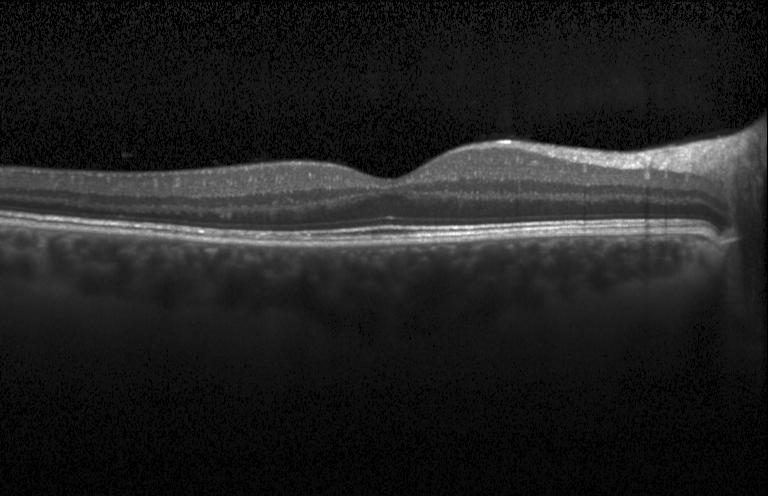 Finding: no choroidal neovascularization, diabetic macular edema, or drusen.